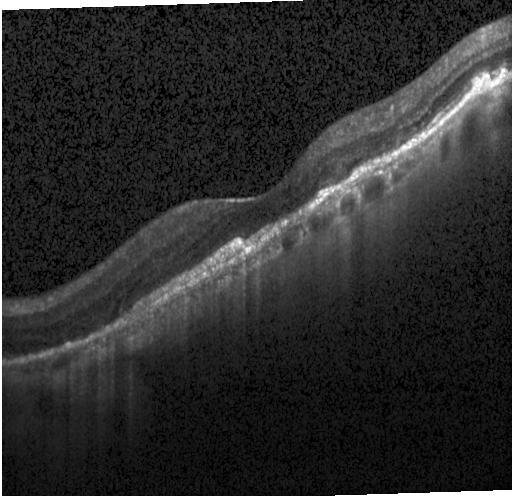

Finding: a choroidal neovascular membrane.